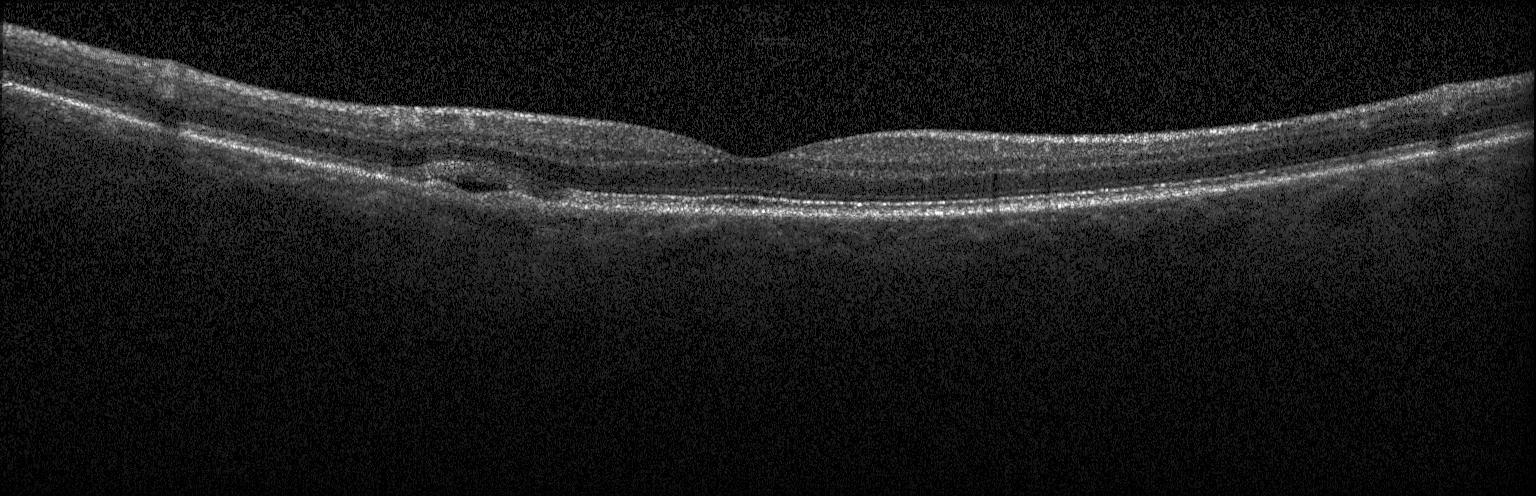 Spectral-domain optical coherence tomography. Optical coherence tomography scan — Impression: a choroidal neovascular membrane.